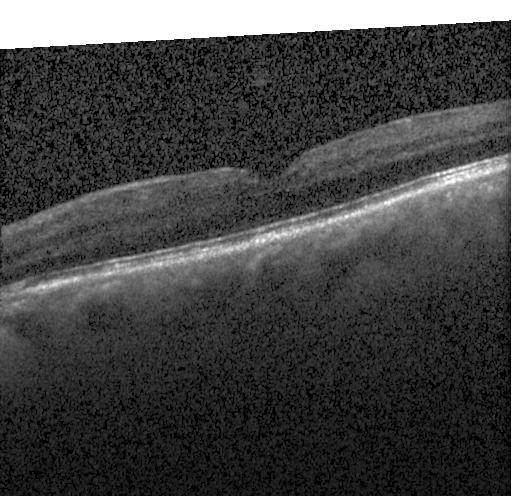

Retinal OCT cross-section. Dx: no choroidal neovascularization, no diabetic macular edema, and no drusen.